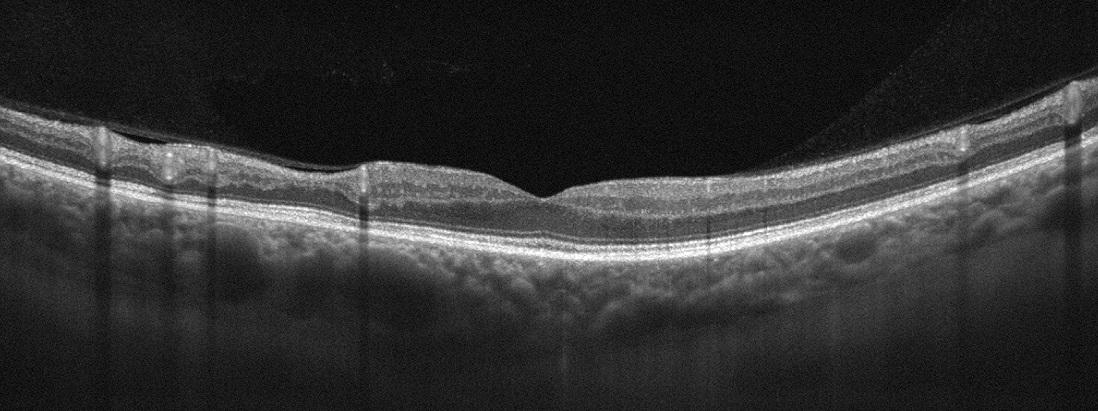
OCT line scan. Assessment: retinal vein occlusion.